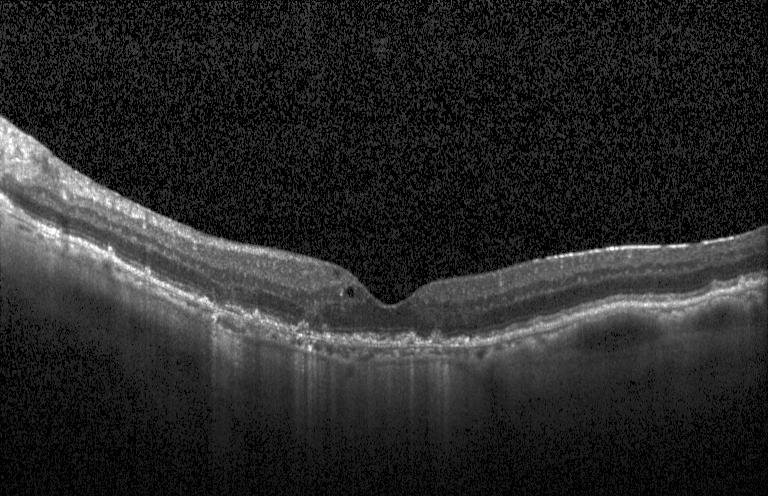
Diagnosis: choroidal neovascularization.